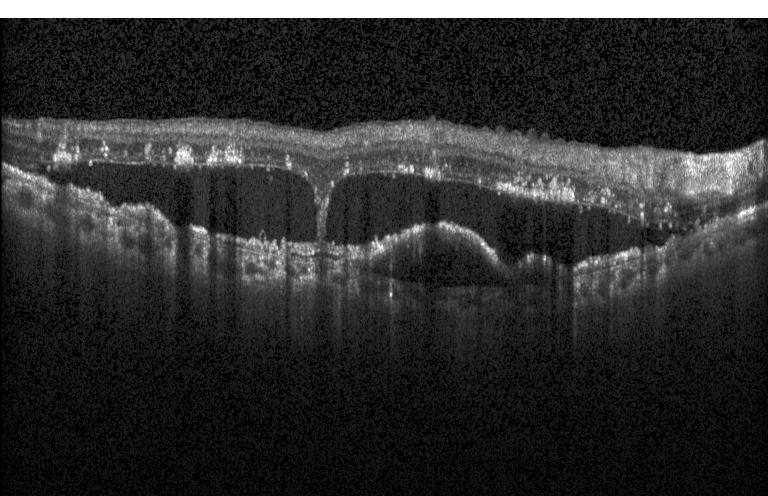
OCT B-scan, SD-OCT, centered on the fovea. Impression: a choroidal neovascular membrane.